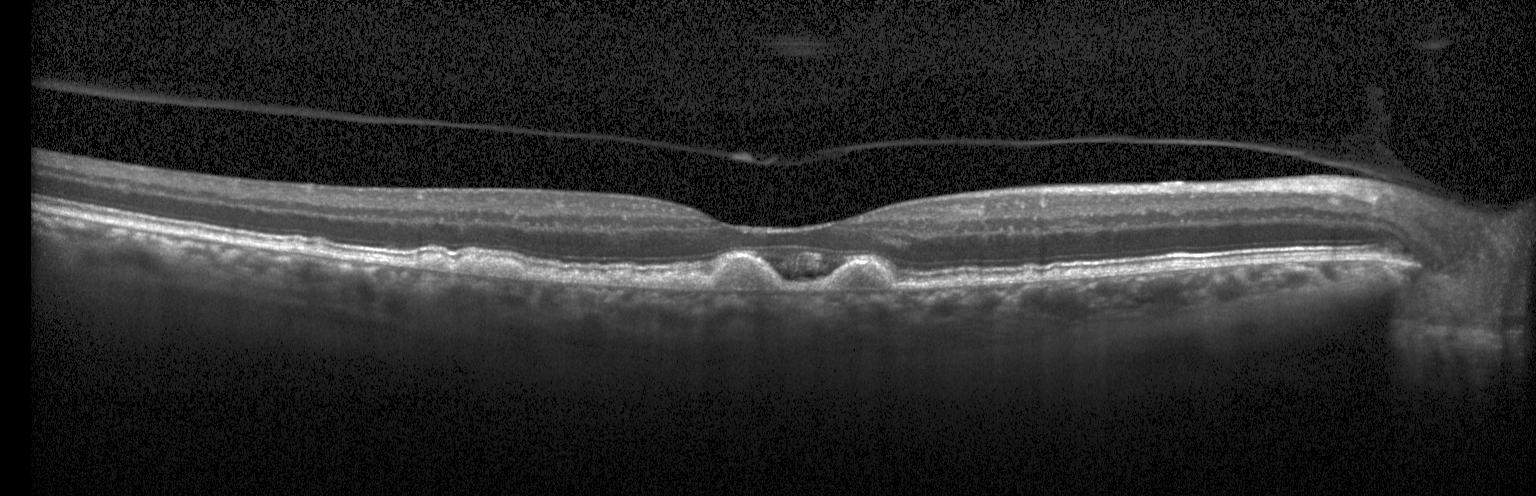

Macular scan · SD-OCT · optical coherence tomography scan. Impression: a choroidal neovascular membrane.